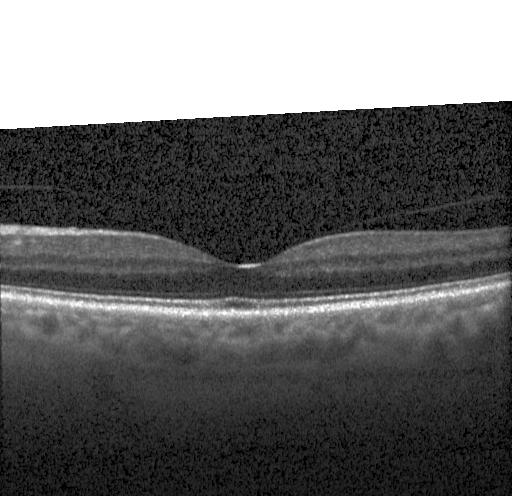
No evidence of CNV, DME, or drusen.